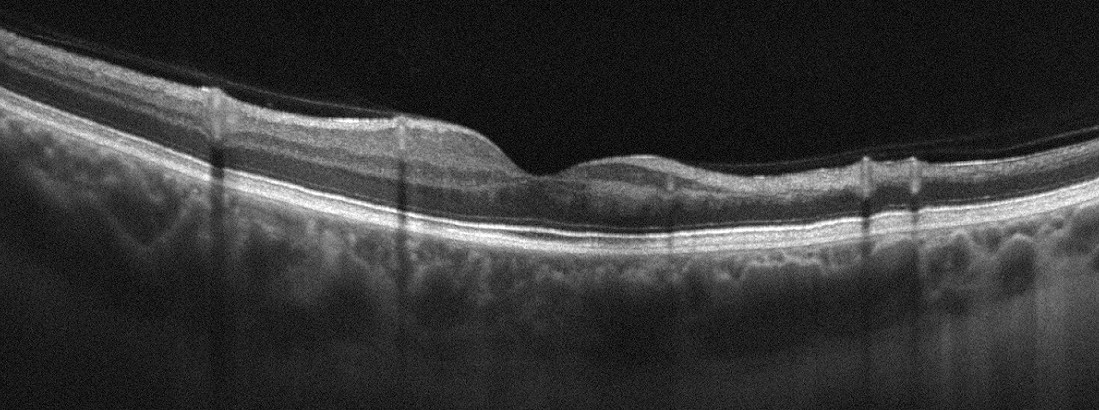

Instrument: Optovue Avanti RTVue XR. Optical coherence tomography scan. Finding: RVO.